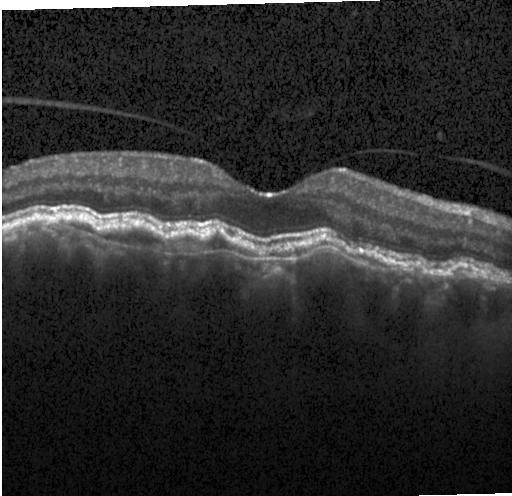
Diagnosis: a choroidal neovascular membrane.